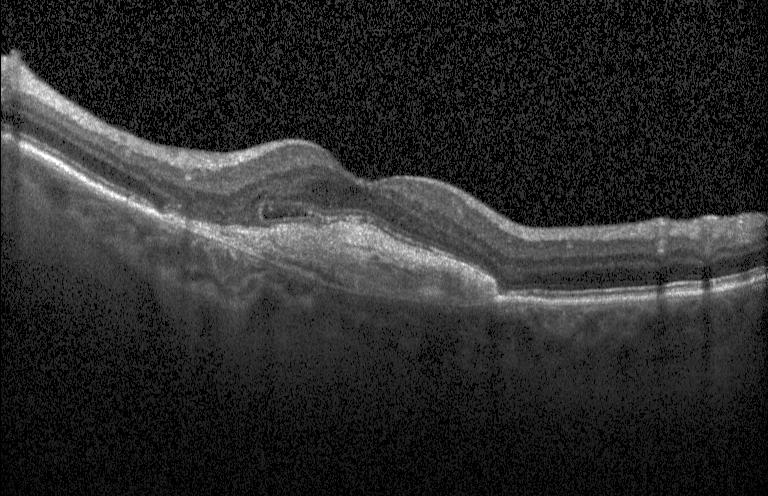

Impression: CNV.